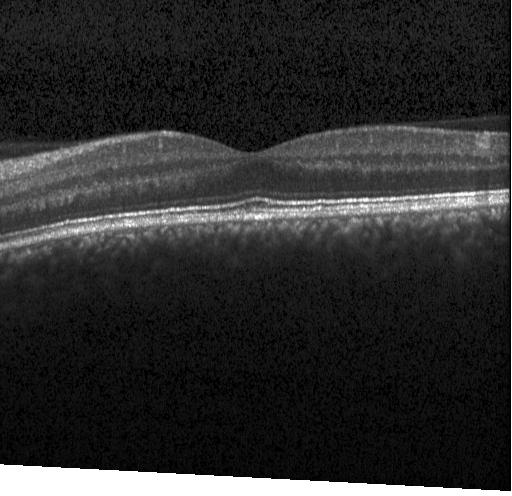
Centered on the fovea, retinal OCT B-scan
The scan shows neither choroidal neovascularization, diabetic macular edema, nor drusen.